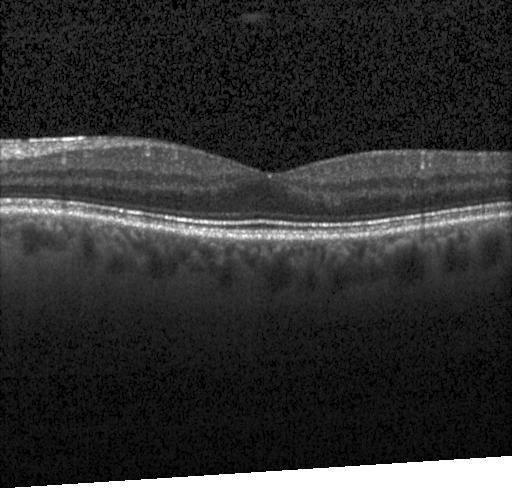

Macular OCT: no choroidal neovascularization, diabetic macular edema, or drusen.